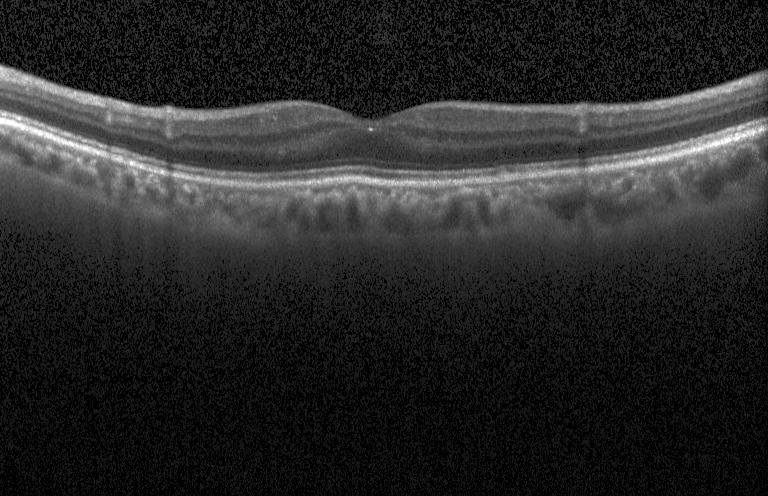

Dx: no choroidal neovascularization, diabetic macular edema, or drusen.